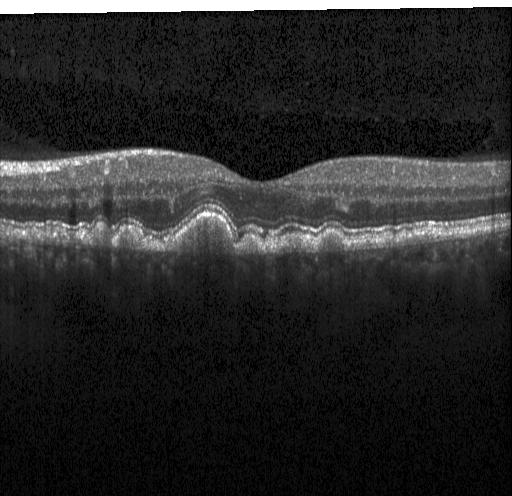

Retinal OCT B-scan — Dx: sub-RPE drusenoid deposits.